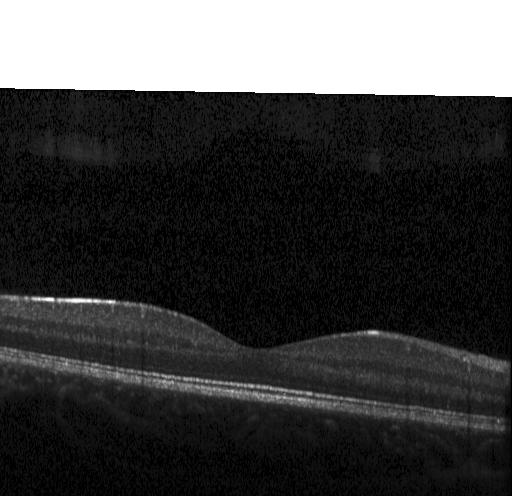
Spectral-domain optical coherence tomography · retinal OCT B-scan — This B-scan demonstrates no evidence of CNV, DME, or drusen.